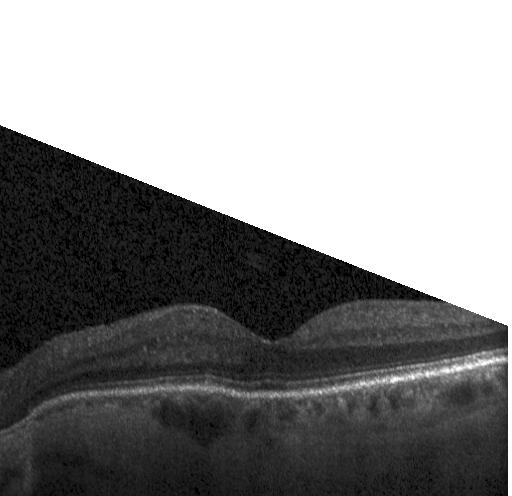 Acquired on a Heidelberg Spectralis, spectral-domain optical coherence tomography, optical coherence tomography B-scan, macular scan. Diagnosis: no choroidal neovascularization, diabetic macular edema, or drusen.